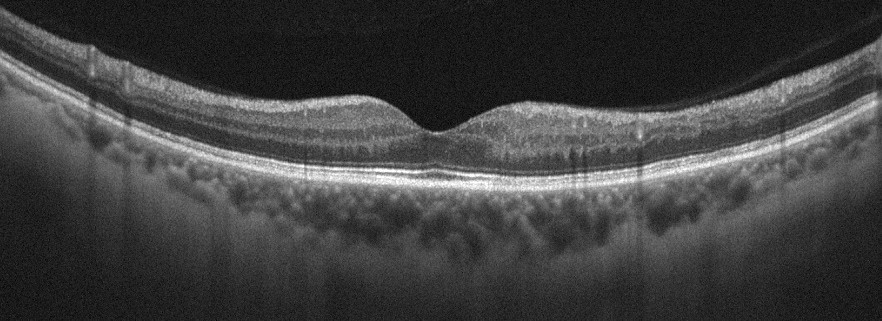 OCT scan showing RVO.